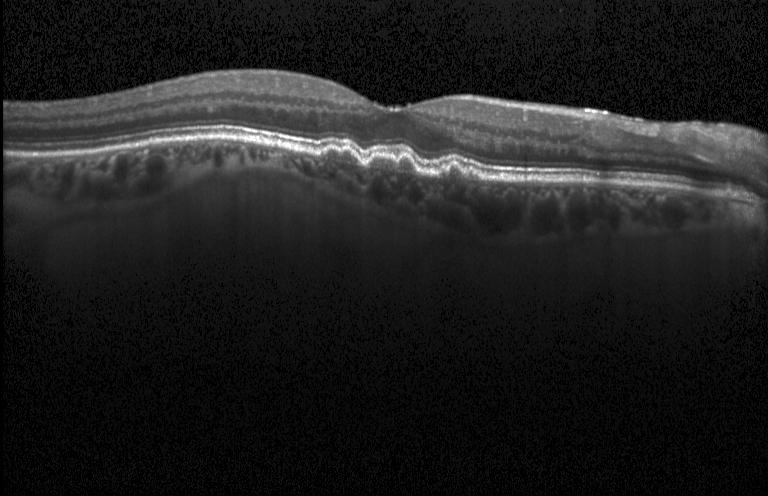

Optical coherence tomography B-scan, through the macula, spectral-domain OCT, instrument: Heidelberg Spectralis — Dx: multiple drusen.